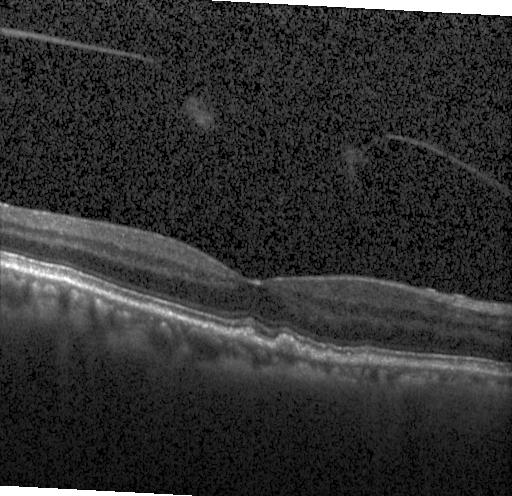 OCT scan showing drusen.